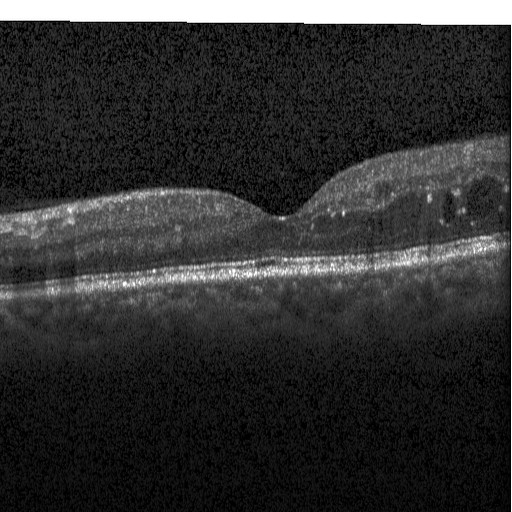

OCT B-scan.
Diagnosis: diabetic macular edema.